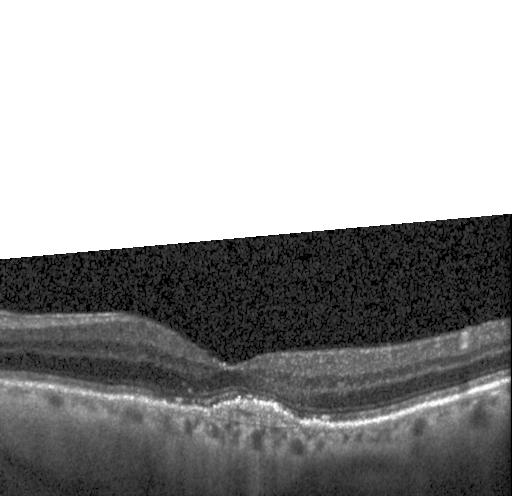
OCT finding: a choroidal neovascular membrane.